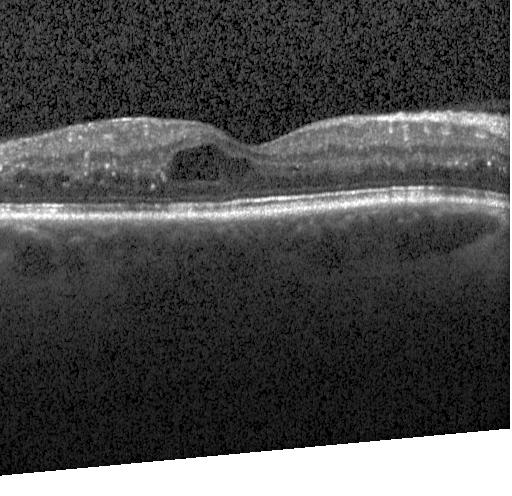

OCT B-scan
Impression: diabetic macular edema.